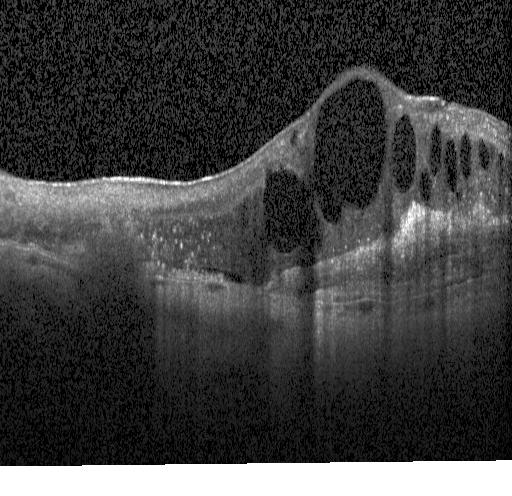
Heidelberg Spectralis OCT system · spectral-domain OCT · through the macula · optical coherence tomography scan.
Assessment: CNV.